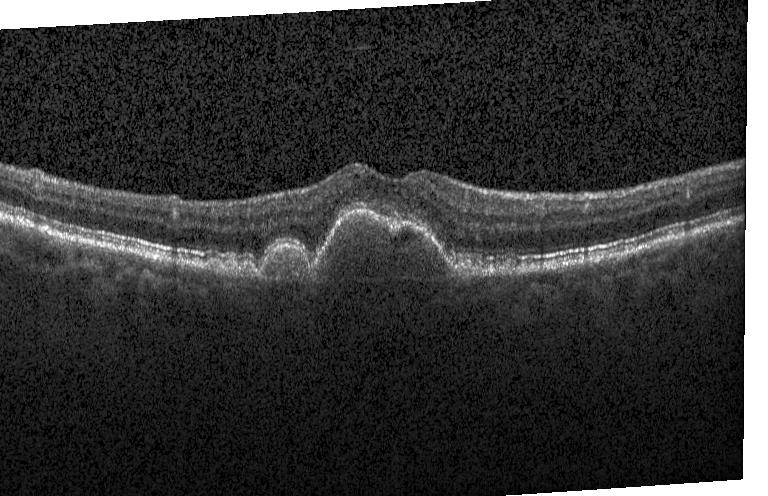
OCT finding: a choroidal neovascular membrane.